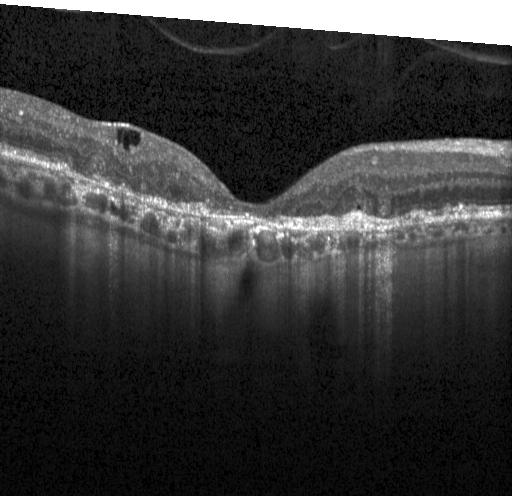
Assessment: a choroidal neovascular membrane.